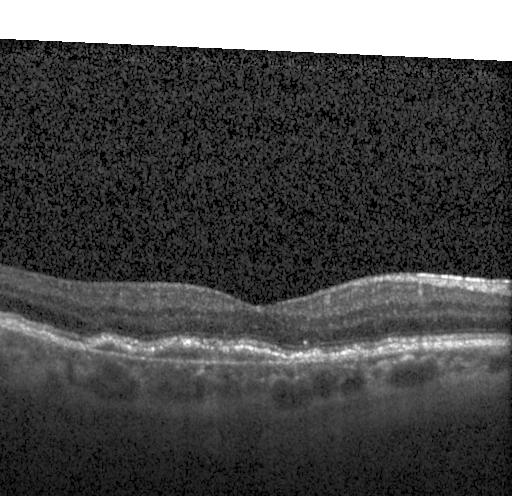
Macular scan · Heidelberg Spectralis · OCT line scan · SD-OCT. Dx: CNV.